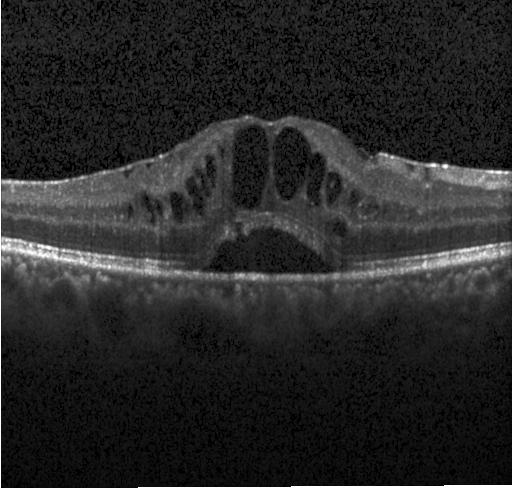
SD-OCT, retinal OCT B-scan. Assessment: diabetic macular edema.